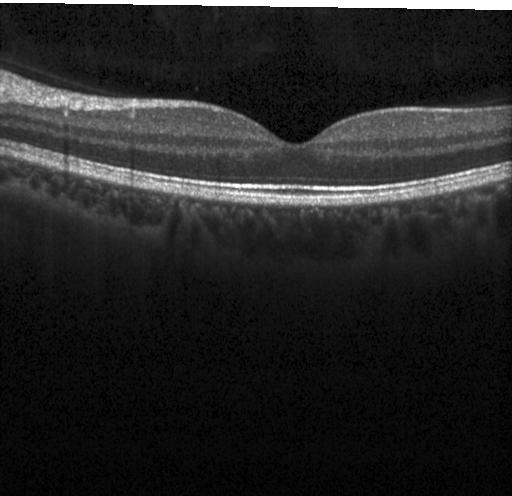
Finding: no CNV, DME, or drusen.